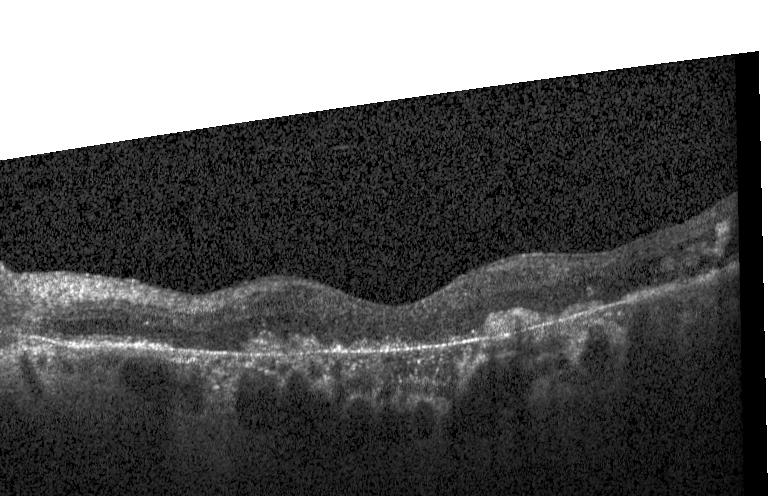 Spectral-domain OCT, optical coherence tomography scan, fovea-centered, acquired on a Heidelberg Spectralis
Impression: a choroidal neovascular membrane.